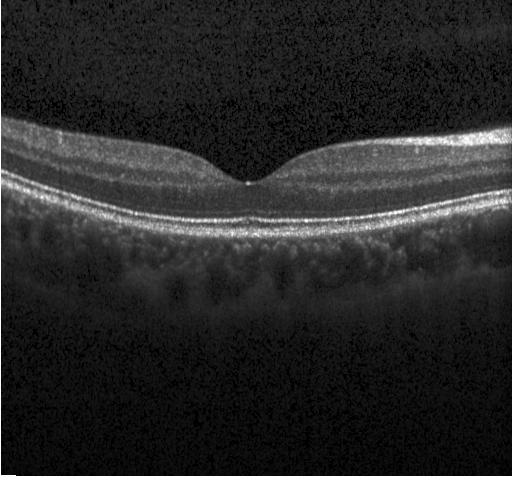

Fovea-centered; optical coherence tomography B-scan
Finding: no evidence of CNV, DME, or drusen.